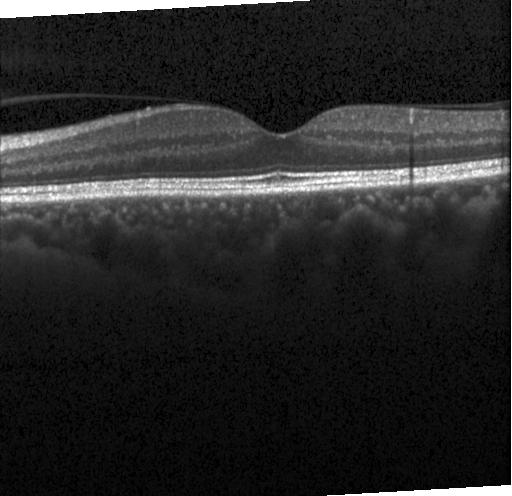

Optical coherence tomography B-scan.
The scan shows neither choroidal neovascularization, diabetic macular edema, nor drusen.